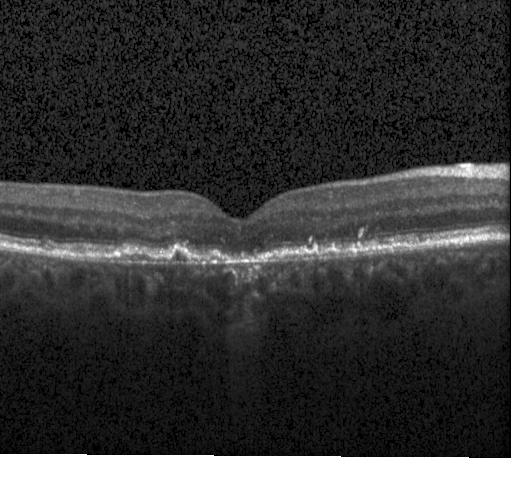

Centered on the fovea. Retinal OCT B-scan. Heidelberg Spectralis. The scan shows CNV.